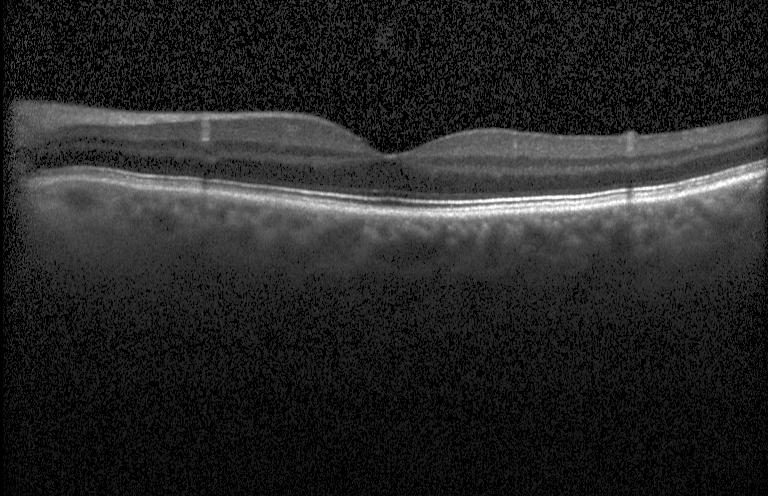

Finding: no choroidal neovascularization, no diabetic macular edema, and no drusen.